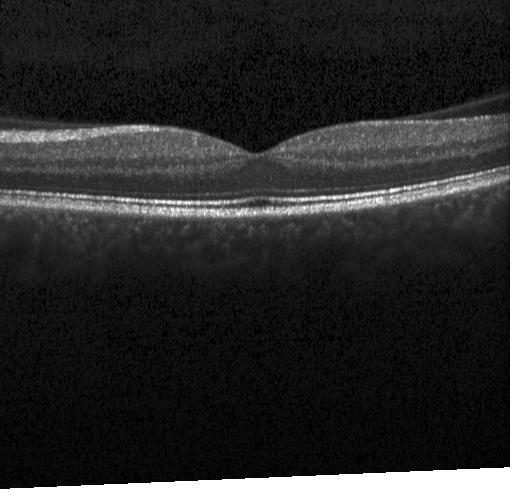
Assessment: no CNV, DME, or drusen.